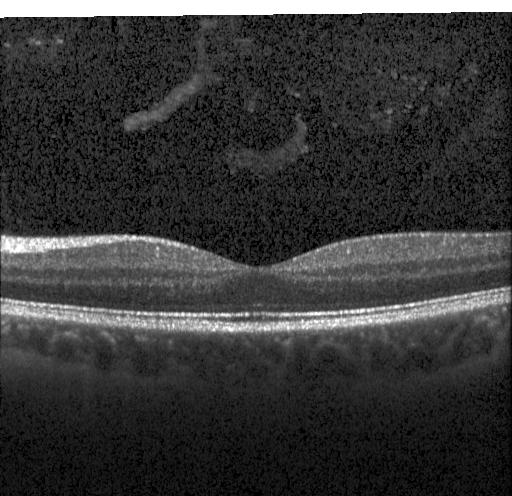 Dx: neither CNV, DME, nor drusen.